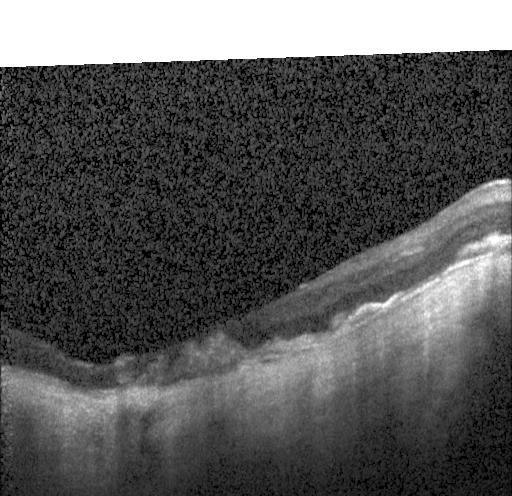
OCT finding: a choroidal neovascular membrane.